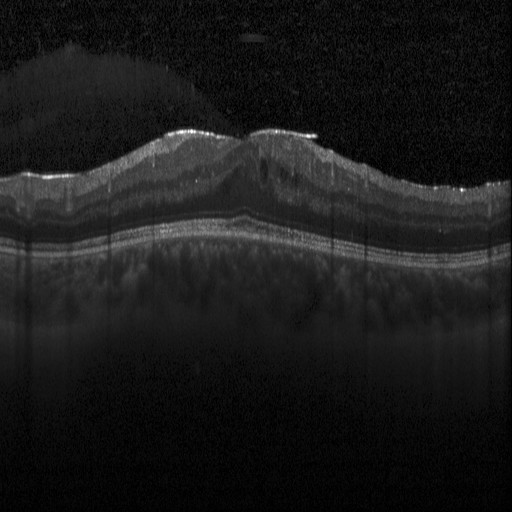

OCT line scan; instrument: Heidelberg Spectralis.
Diagnosis: DME.